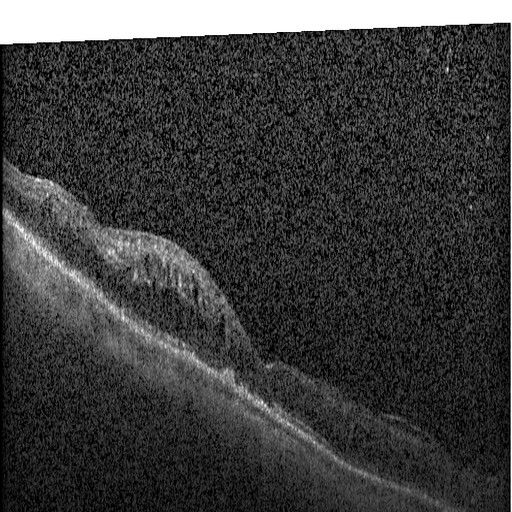

OCT B-scan showing DME.